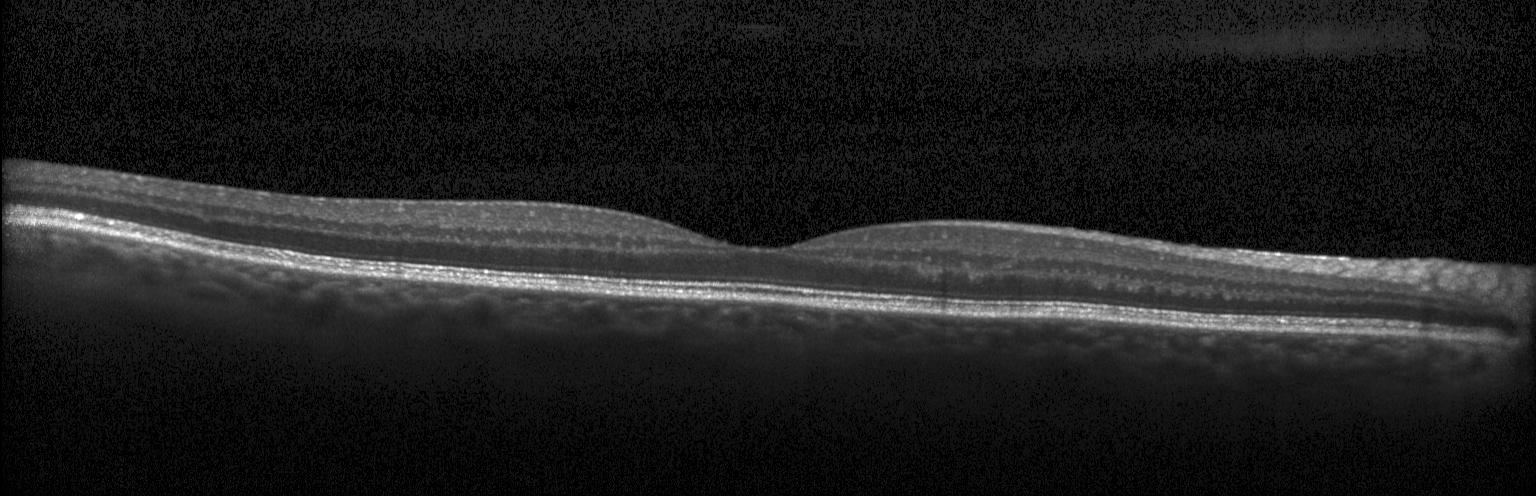

Retinal OCT B-scan. Assessment: no CNV, DME, or drusen.